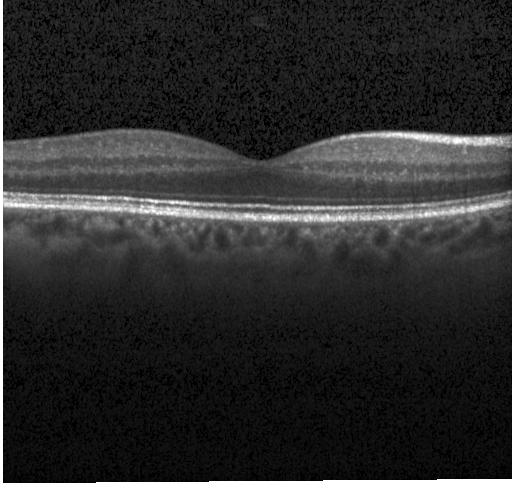

Heidelberg Spectralis OCT system · SD-OCT · optical coherence tomography B-scan · through the macula. Diagnosis: neither choroidal neovascularization, diabetic macular edema, nor drusen.